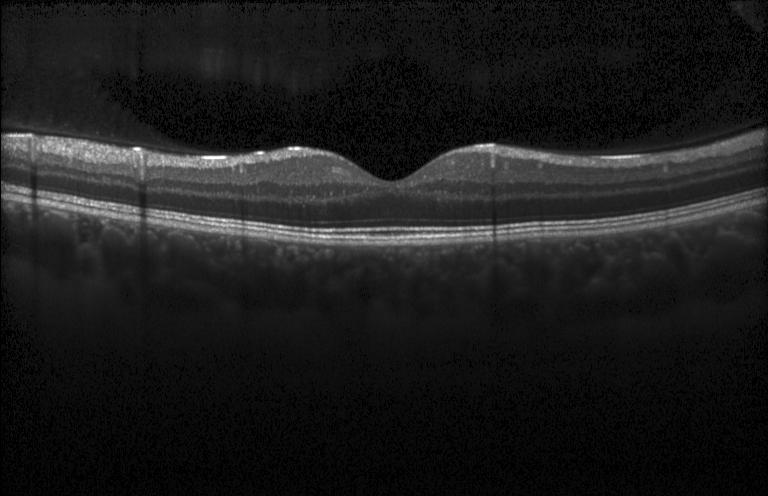
Heidelberg Spectralis. Optical coherence tomography scan. Spectral-domain optical coherence tomography. Finding: no choroidal neovascularization, no diabetic macular edema, and no drusen.